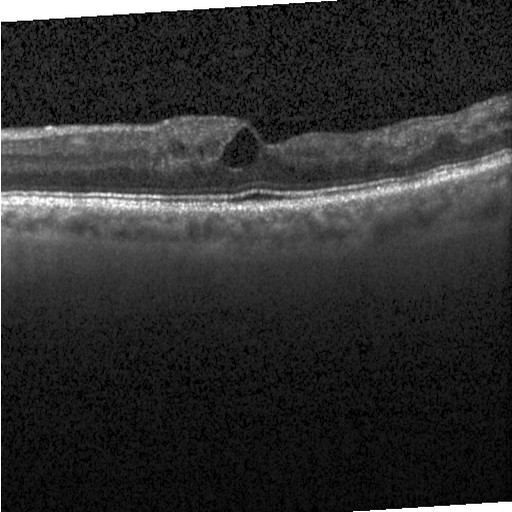

Retinal OCT B-scan — OCT finding: diabetic macular edema.